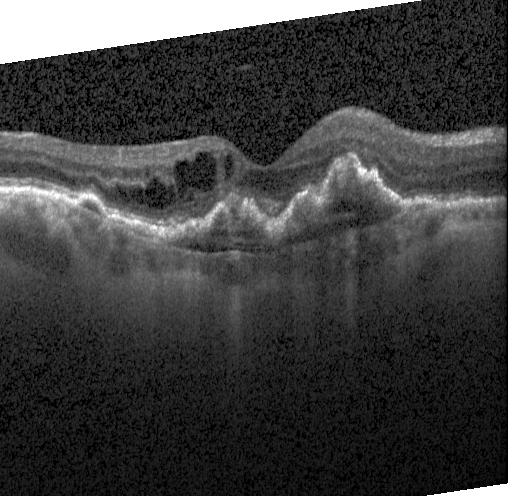 Optical coherence tomography scan. Dx: choroidal neovascularization (CNV).